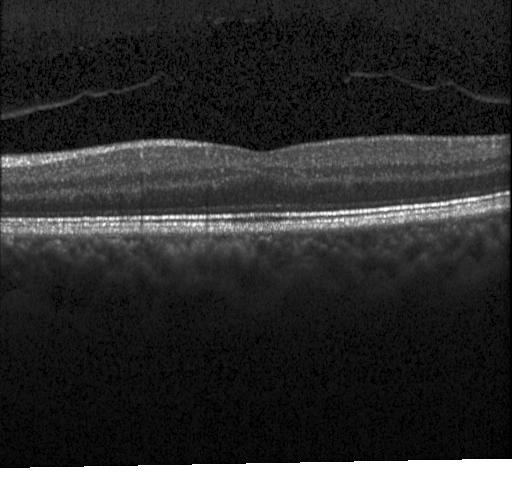

Retinal OCT cross-section.
No choroidal neovascularization, no diabetic macular edema, and no drusen.